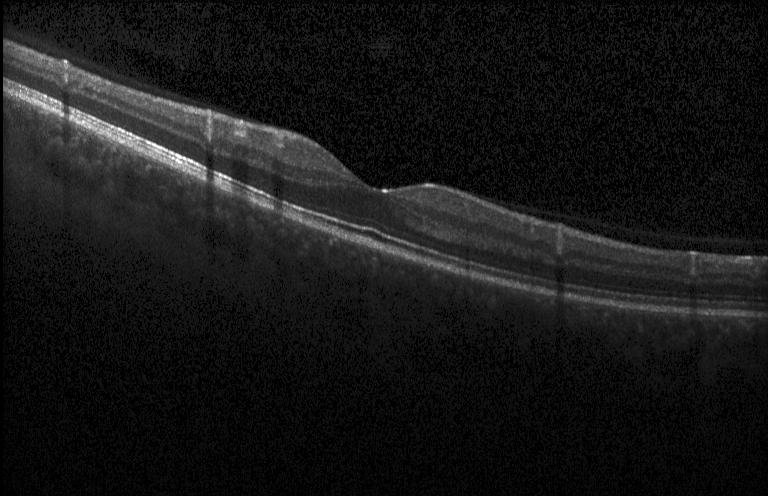
Optical coherence tomography scan.
Finding: no choroidal neovascularization, no diabetic macular edema, and no drusen.